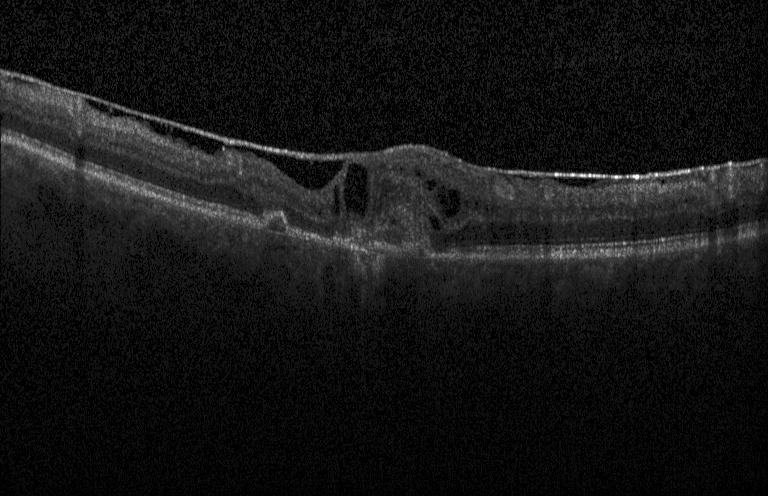 Acquired on a Heidelberg Spectralis, SD-OCT, optical coherence tomography B-scan
CNV.